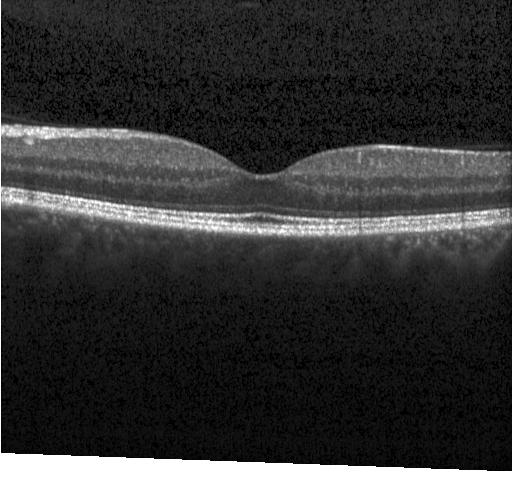

OCT B-scan. Centered on the fovea. Dx: neither choroidal neovascularization, diabetic macular edema, nor drusen.